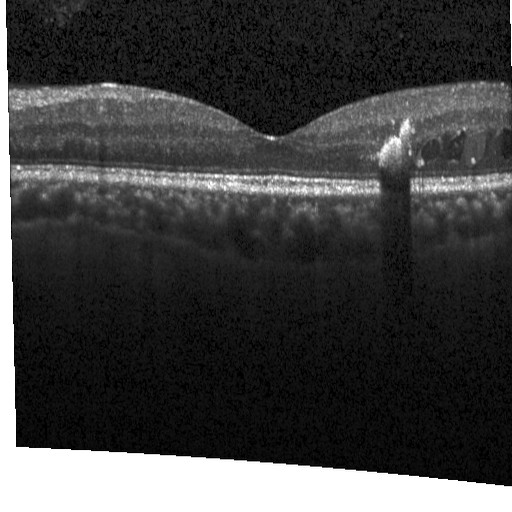
OCT line scan. Impression: DME.